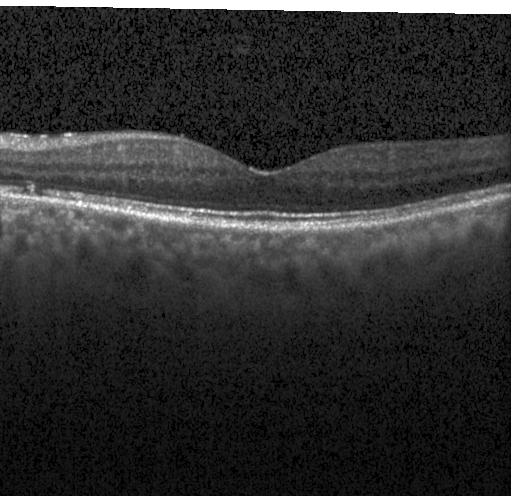

Through the macula · instrument: Heidelberg Spectralis · optical coherence tomography scan — Dx: no choroidal neovascularization, no diabetic macular edema, and no drusen.